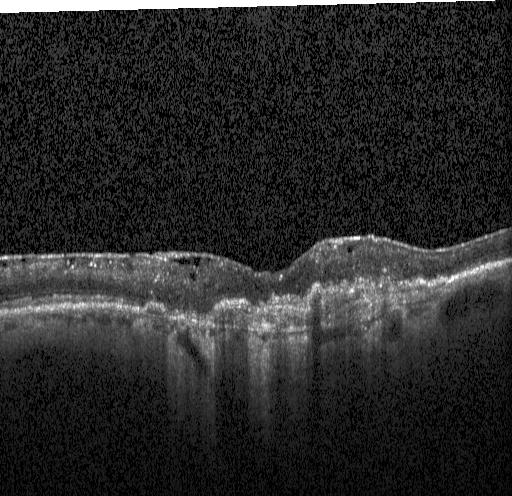 Impression: choroidal neovascularization (CNV).